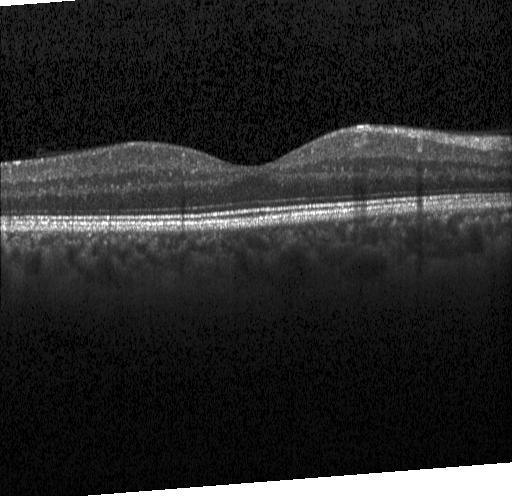

OCT B-scan
Diagnosis: neither choroidal neovascularization, diabetic macular edema, nor drusen.